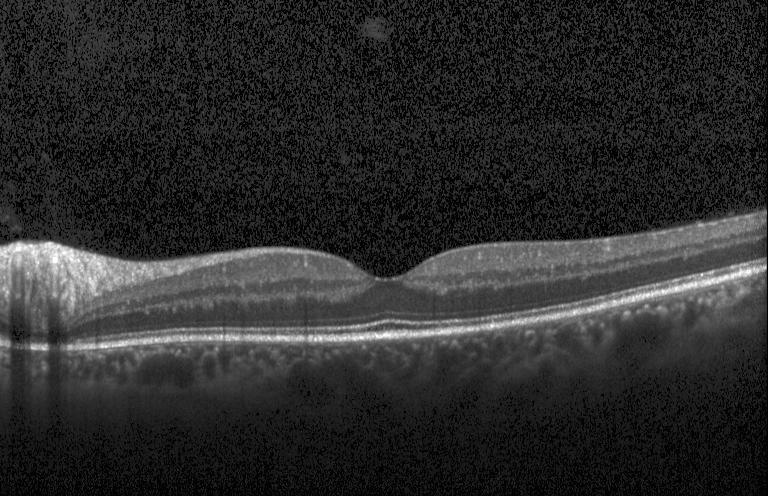

Macular OCT: neither CNV, DME, nor drusen.